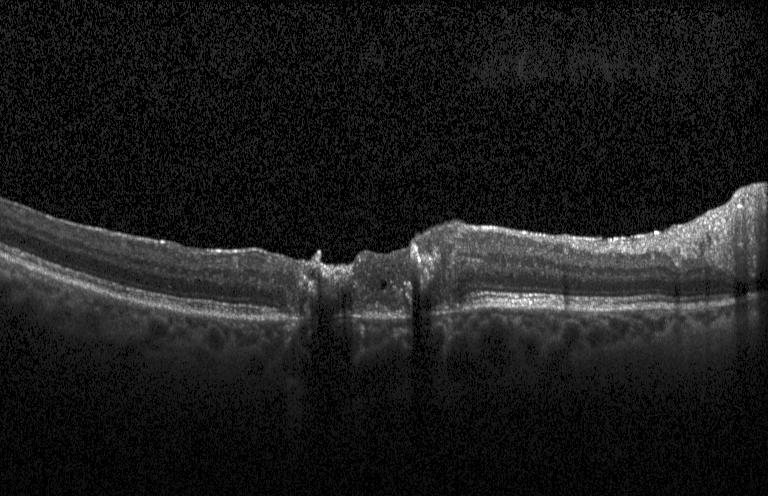 Macular OCT demonstrating a choroidal neovascular membrane.